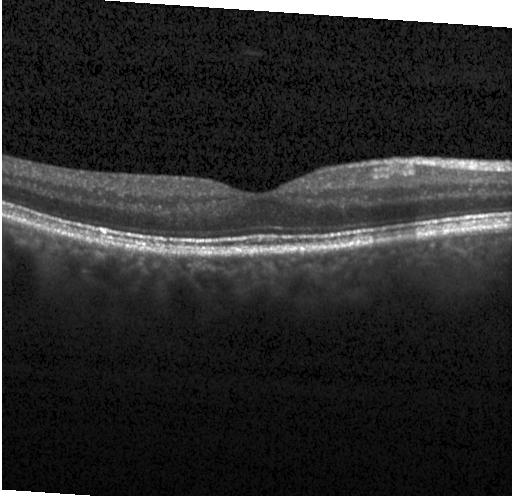
Retinal OCT cross-section showing no CNV, no DME, and no drusen.